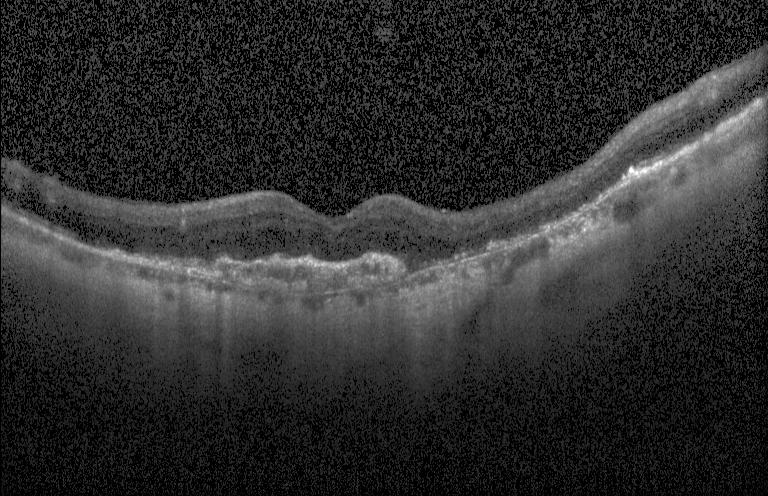
Acquired on a Heidelberg Spectralis; optical coherence tomography scan; spectral-domain OCT; macular scan
The scan shows CNV.